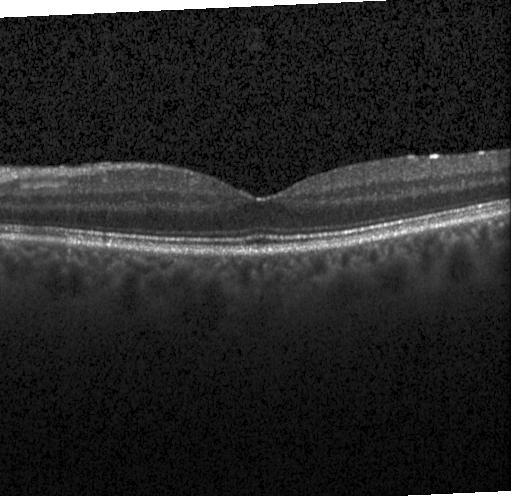 Diagnosis: no choroidal neovascularization, no diabetic macular edema, and no drusen.